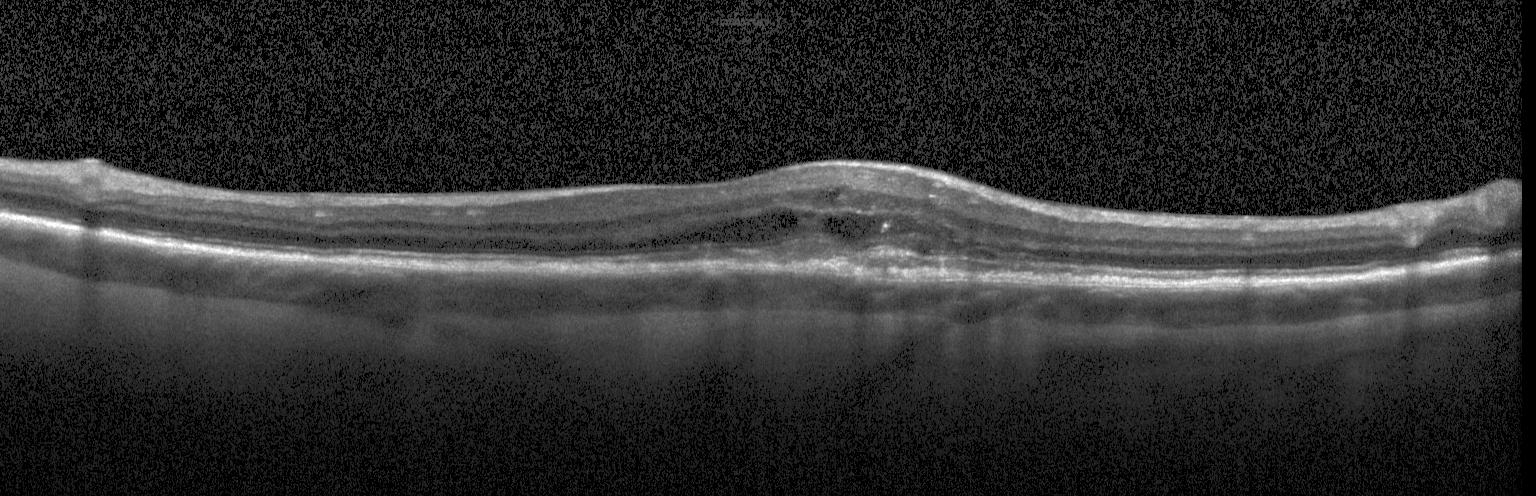
Optical coherence tomography B-scan.
Finding: a choroidal neovascular membrane.